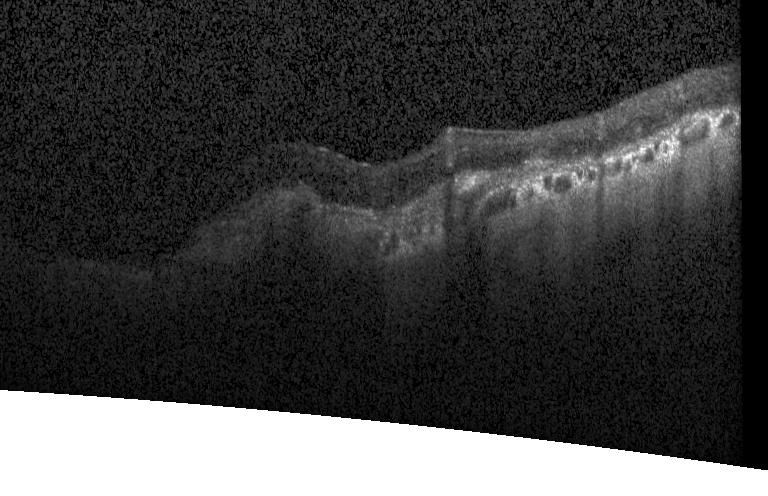

OCT line scan · macular scan. A choroidal neovascular membrane.